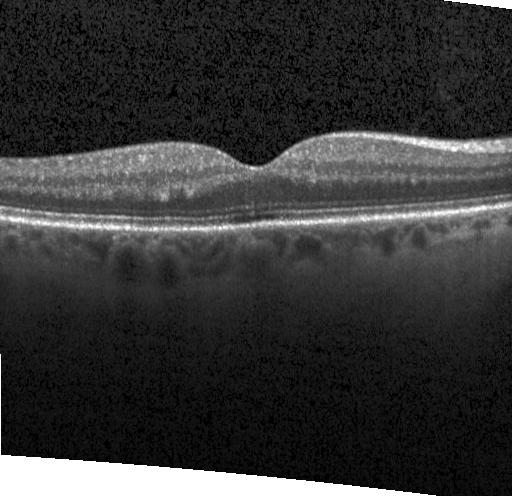

OCT scan showing neither choroidal neovascularization, diabetic macular edema, nor drusen.